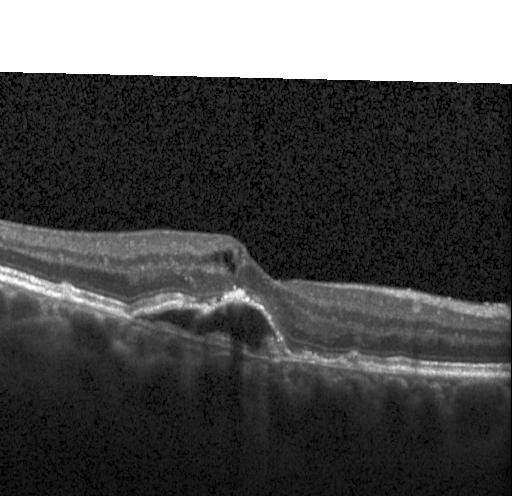 Retinal OCT cross-section, spectral-domain optical coherence tomography
Diagnosis: CNV.